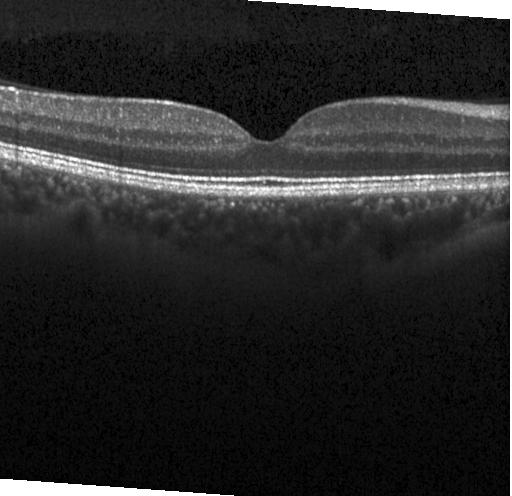
Macular OCT demonstrating no choroidal neovascularization, diabetic macular edema, or drusen.